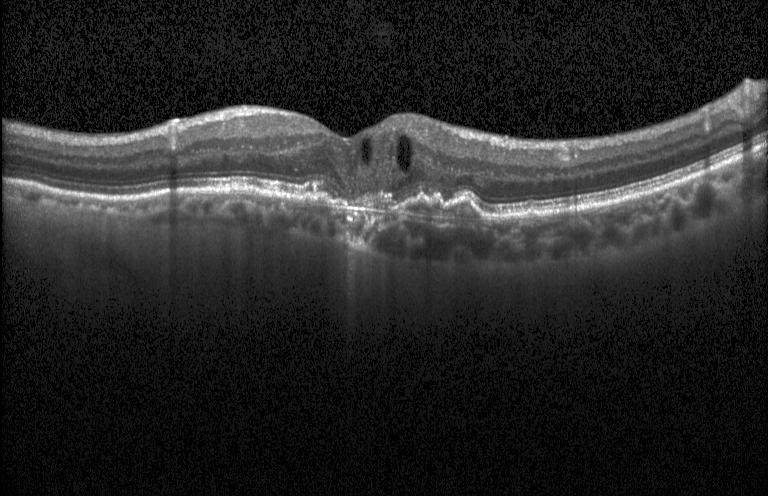

Retinal OCT cross-section. Spectral-domain OCT — OCT finding: a choroidal neovascular membrane.